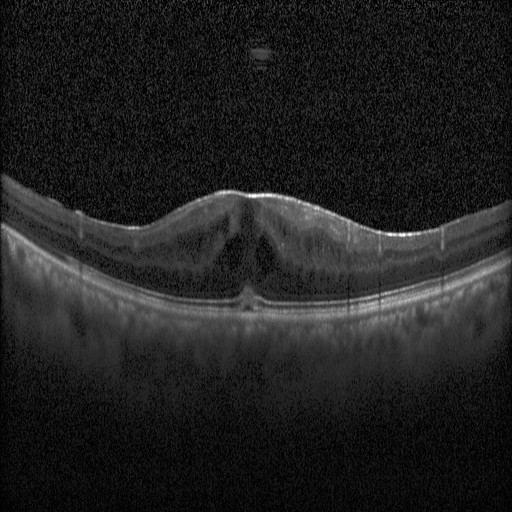

Dx: diabetic macular edema.